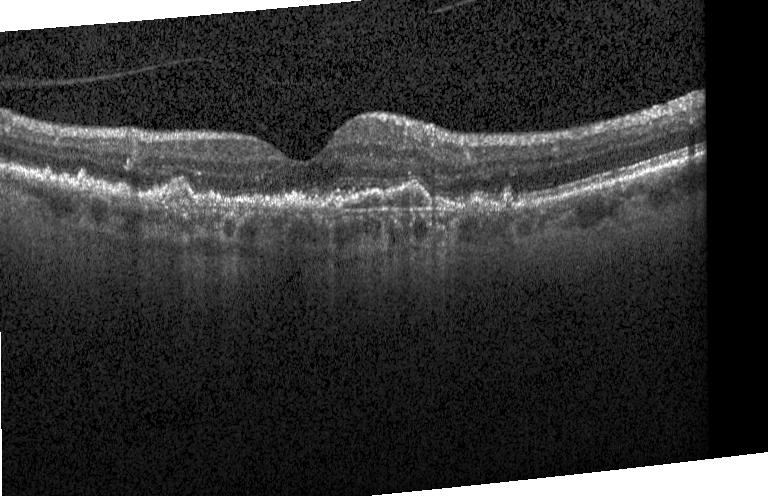

Diagnosis: a choroidal neovascular membrane.